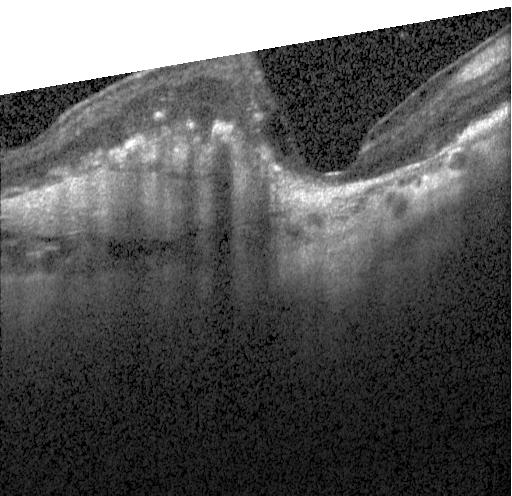 Diagnosis: CNV.